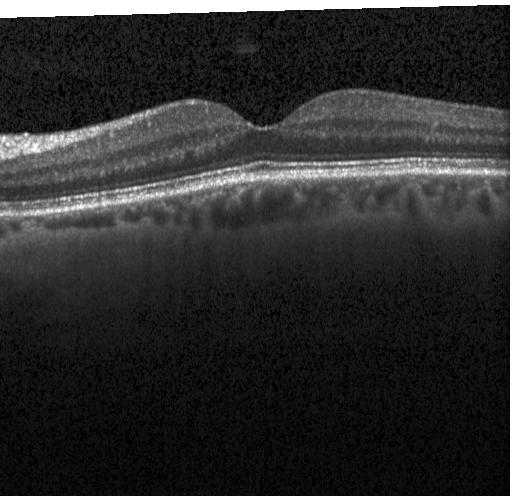
Retinal OCT cross-section · Heidelberg Spectralis OCT system · macular scan. Finding: no CNV, no DME, and no drusen.